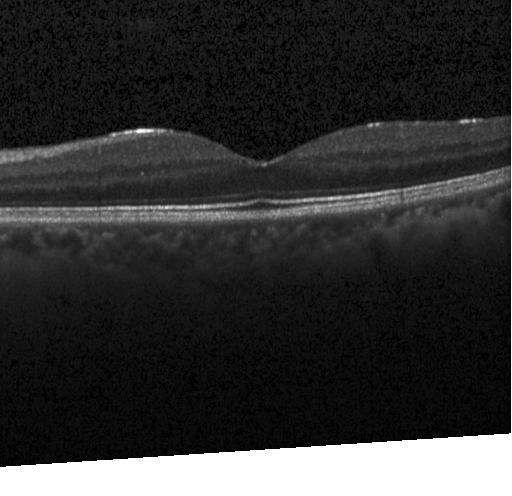
This B-scan demonstrates neither CNV, DME, nor drusen.